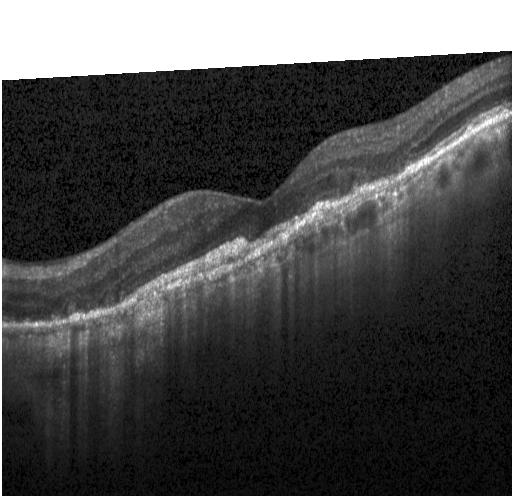

Horizontal scan through the fovea · OCT B-scan.
Finding: choroidal neovascularization (CNV).